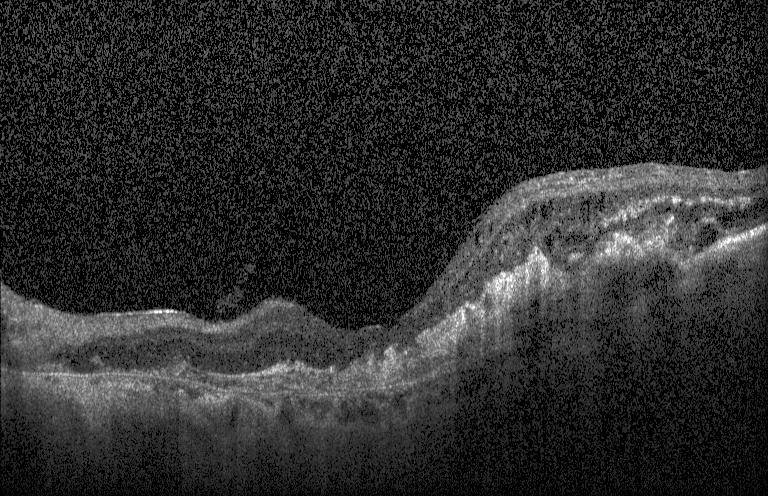

OCT B-scan; through the macula; spectral-domain OCT; instrument: Heidelberg Spectralis.
Finding: a choroidal neovascular membrane.